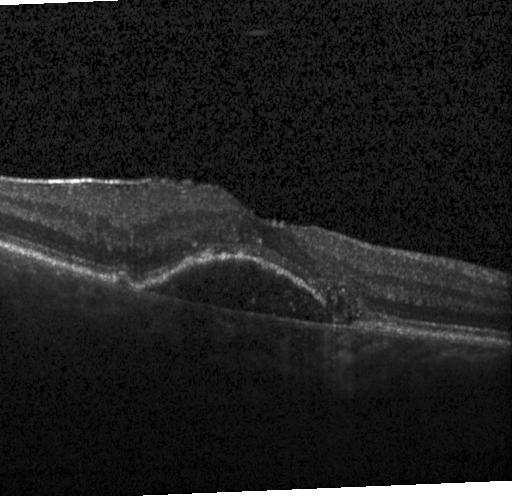

Retinal OCT B-scan.
Diagnosis: a choroidal neovascular membrane.